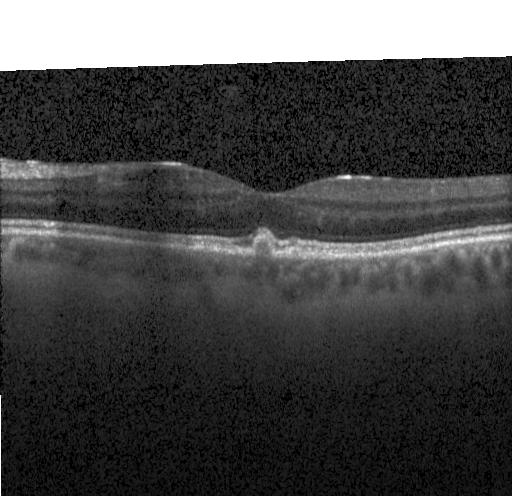

Optical coherence tomography scan, spectral-domain OCT, acquired on a Heidelberg Spectralis.
Finding: drusen.